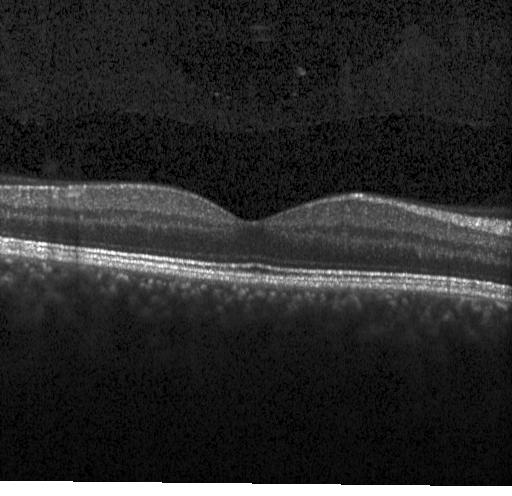 OCT line scan. Heidelberg Spectralis. Spectral-domain optical coherence tomography. Macular scan. Impression: neither CNV, DME, nor drusen.